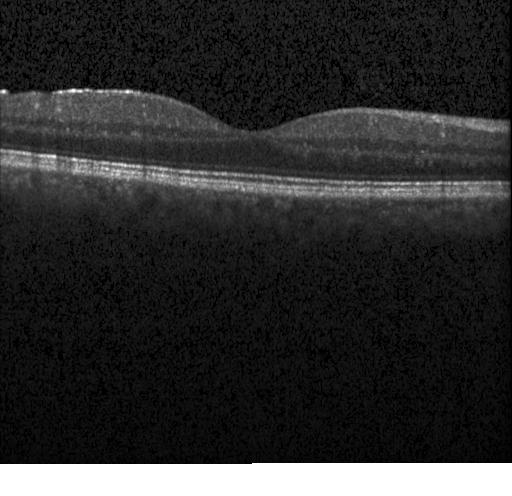 Diagnosis: no CNV, DME, or drusen.